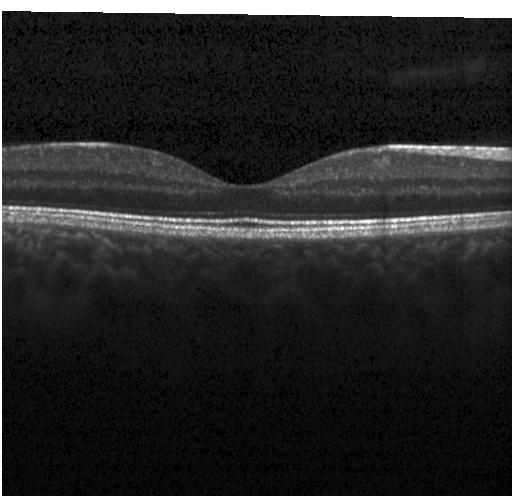 Instrument: Heidelberg Spectralis, OCT line scan, spectral-domain OCT
Diagnosis: no evidence of choroidal neovascularization, diabetic macular edema, or drusen.